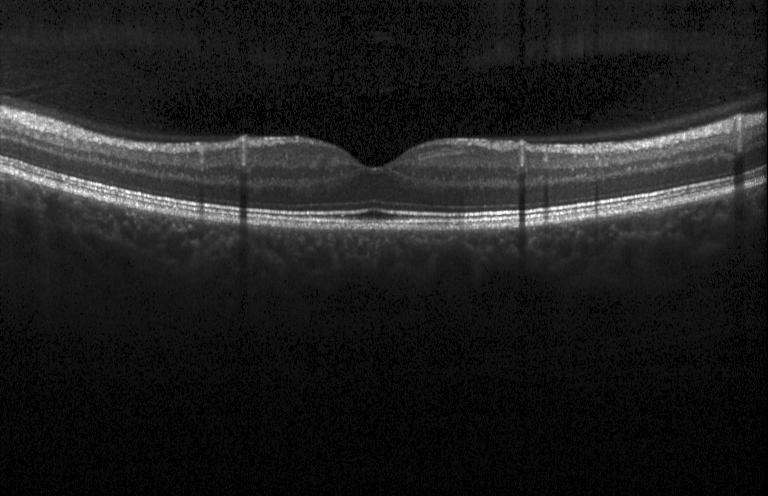

Diagnosis: no evidence of CNV, DME, or drusen.